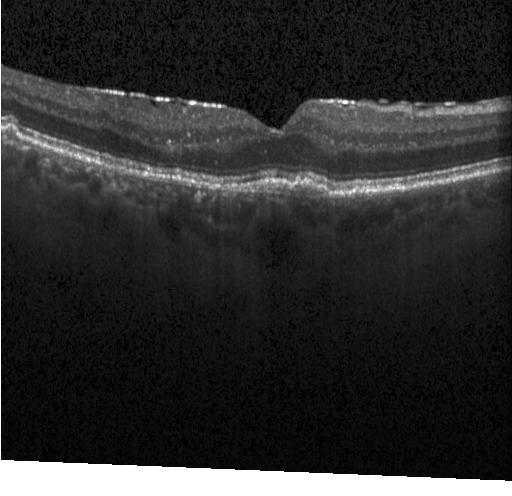

Retinal OCT B-scan.
Impression: a choroidal neovascular membrane.